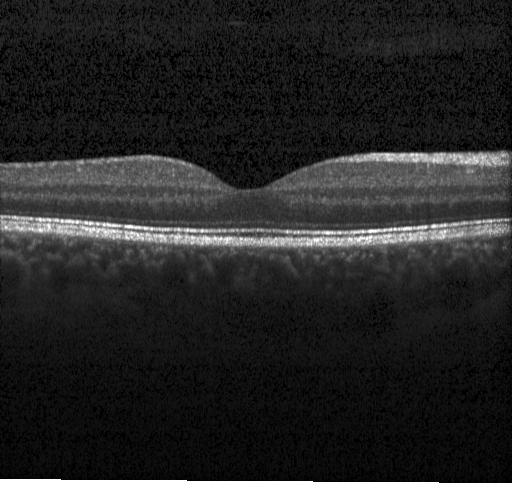

Macular OCT: no CNV, no DME, and no drusen.